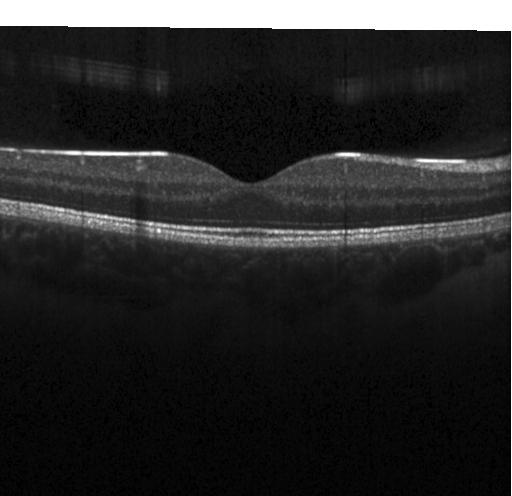
Macular OCT: no CNV, no DME, and no drusen.